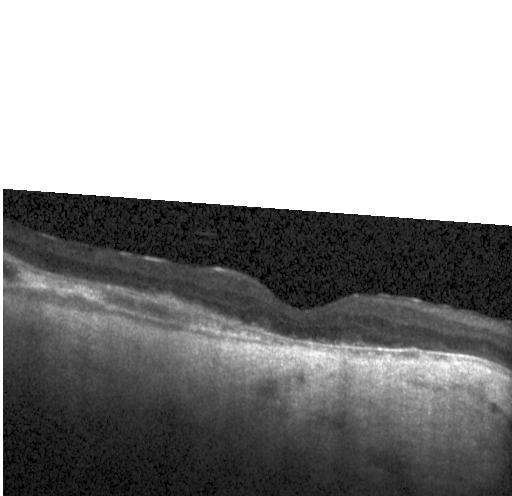 OCT line scan · acquired on a Heidelberg Spectralis · fovea-centered · spectral-domain optical coherence tomography
Impression: CNV.